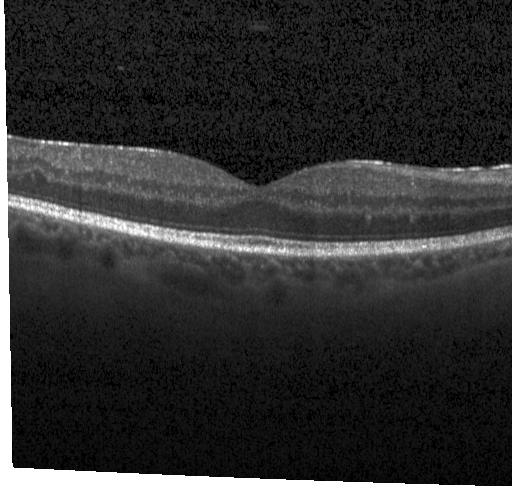
This B-scan demonstrates neither CNV, DME, nor drusen.